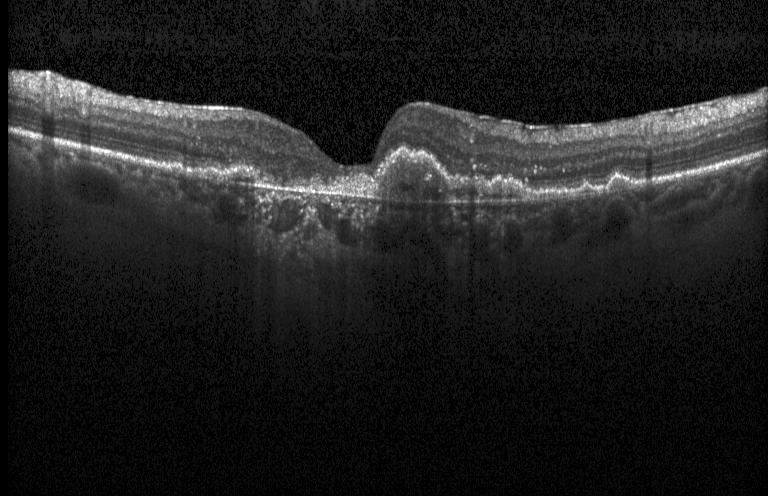
Spectral-domain optical coherence tomography · OCT B-scan · Heidelberg Spectralis.
Finding: a choroidal neovascular membrane.